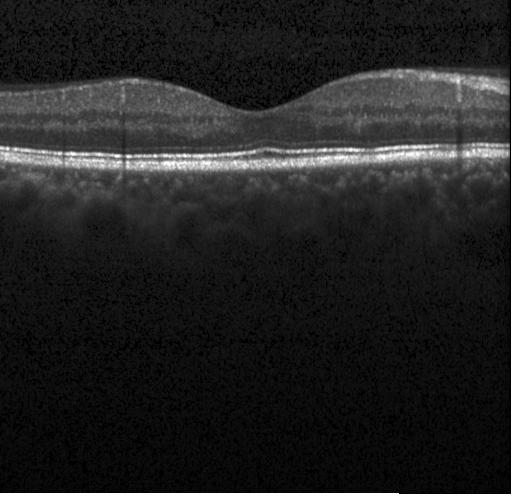 Through the macula · SD-OCT · OCT line scan.
Impression: no CNV, no DME, and no drusen.